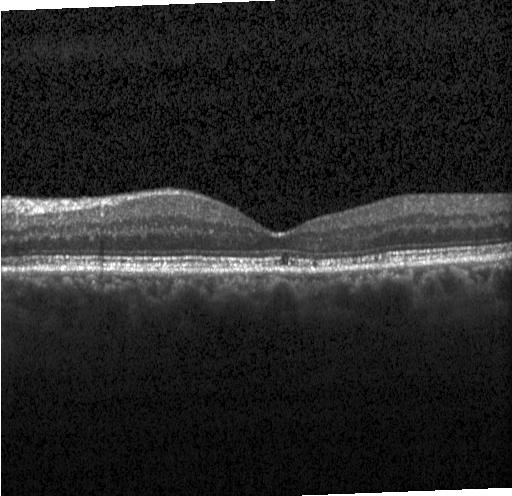
Dx: no evidence of choroidal neovascularization, diabetic macular edema, or drusen.